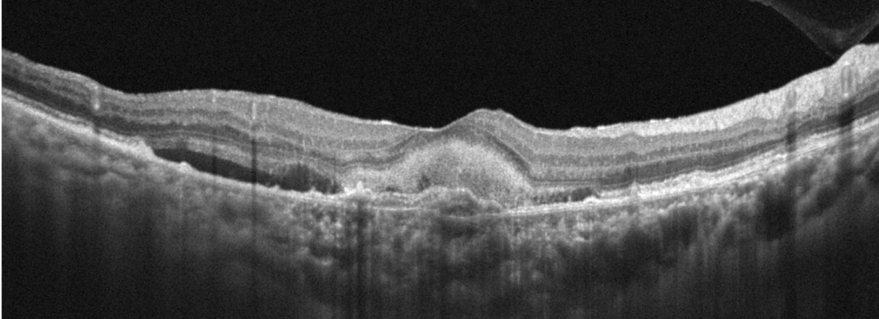 Optical coherence tomography B-scan — Impression: age-related macular degeneration.